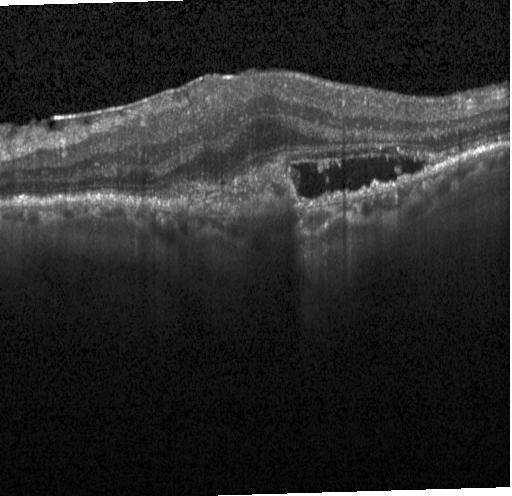
Heidelberg Spectralis OCT system. Spectral-domain OCT. Optical coherence tomography scan. Centered on the fovea. Impression: a choroidal neovascular membrane.